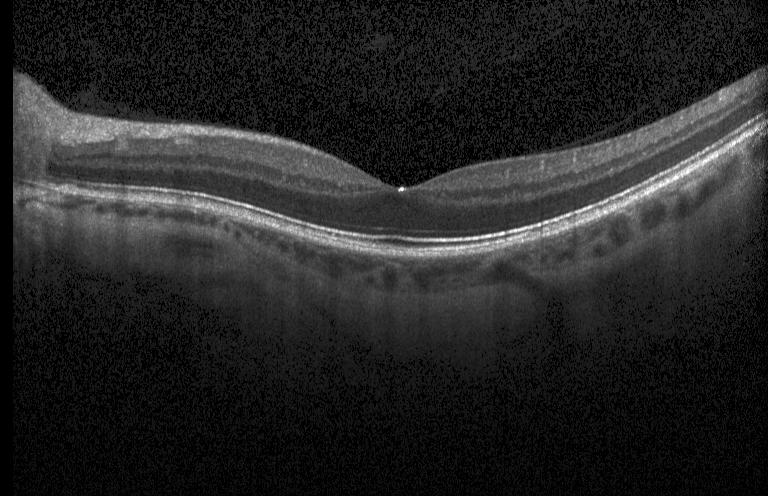
Assessment: no evidence of choroidal neovascularization, diabetic macular edema, or drusen.